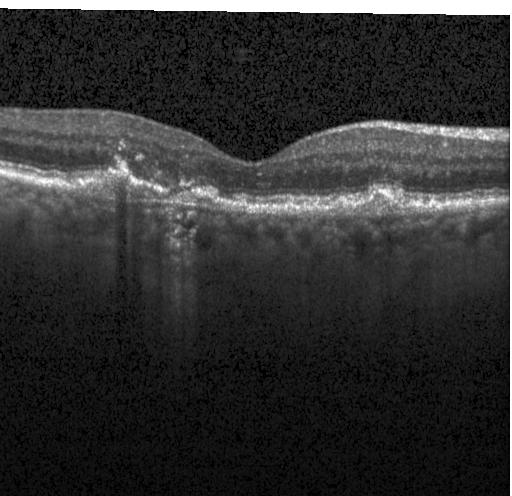 Spectral-domain OCT B-scan: a choroidal neovascular membrane.